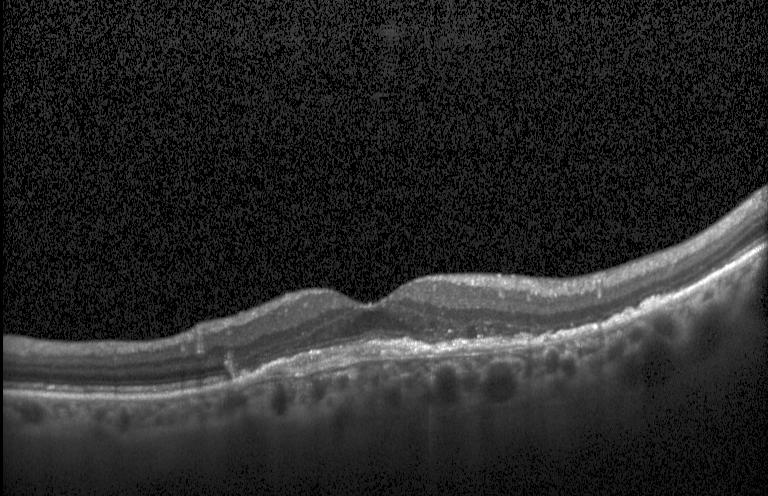 OCT B-scan showing choroidal neovascularization.